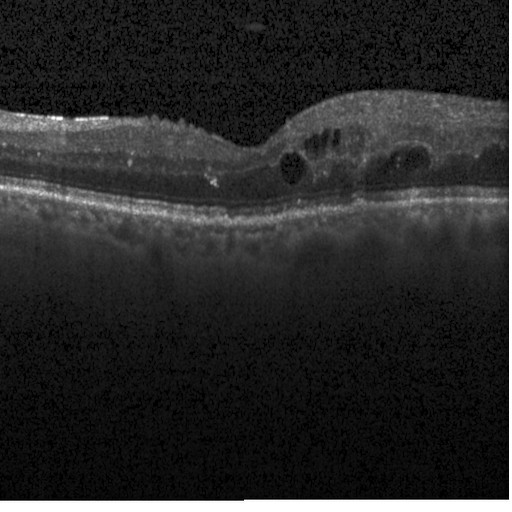 OCT scan showing diabetic macular edema.